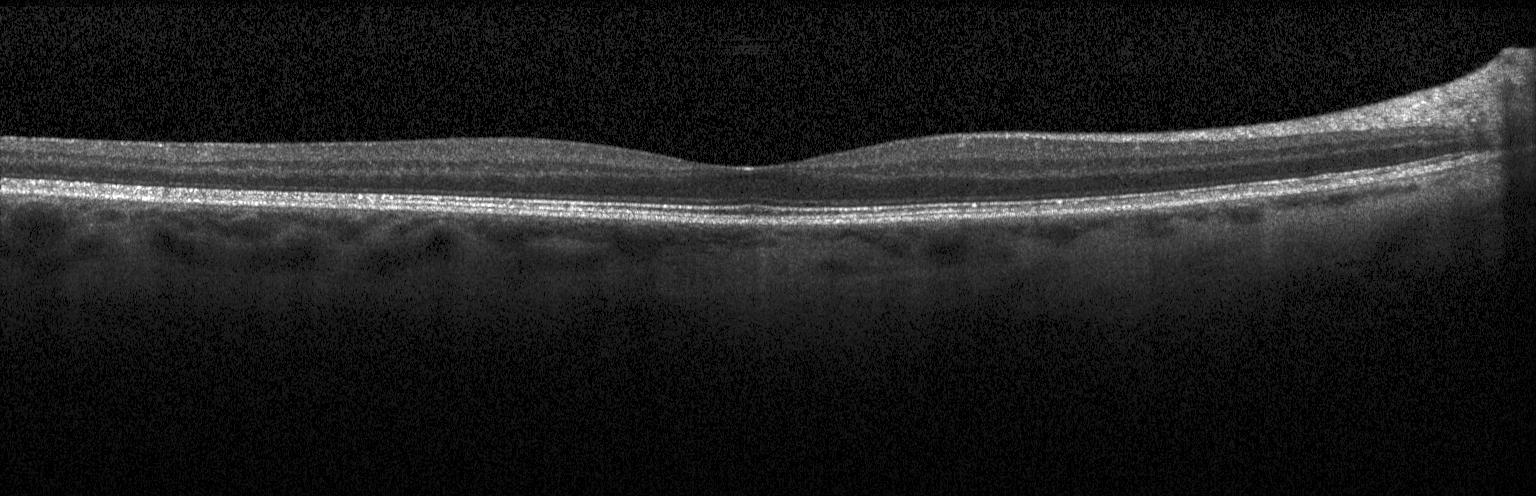 Diagnosis: no choroidal neovascularization, no diabetic macular edema, and no drusen.